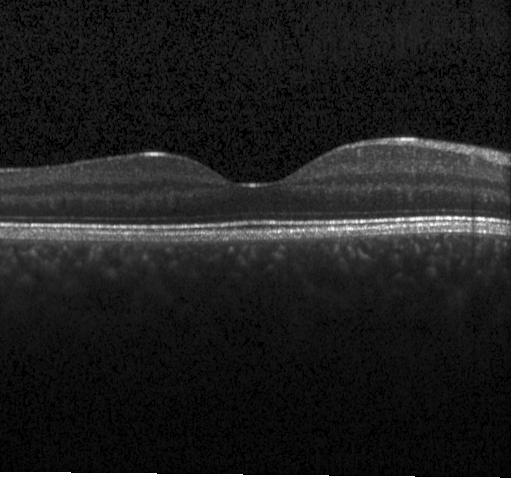 Centered on the fovea; OCT line scan — Impression: neither choroidal neovascularization, diabetic macular edema, nor drusen.